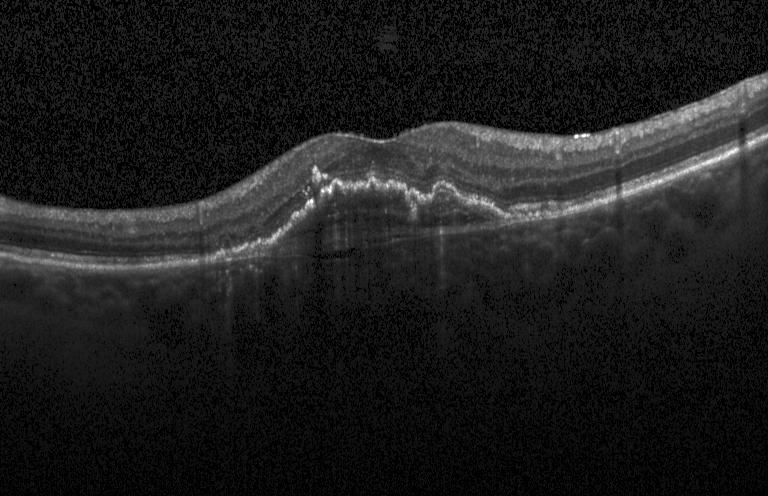

Assessment: choroidal neovascularization (CNV).